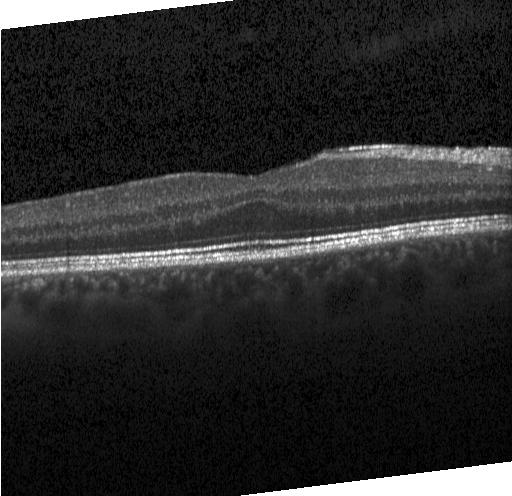 Spectral-domain optical coherence tomography, fovea-centered, retinal OCT B-scan, Heidelberg Spectralis. Impression: neither choroidal neovascularization, diabetic macular edema, nor drusen.